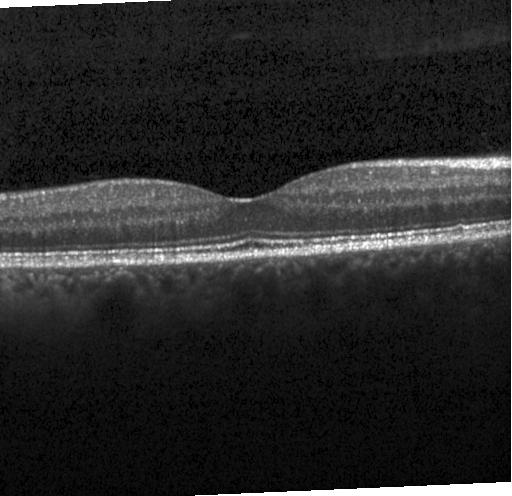
OCT line scan, instrument: Heidelberg Spectralis.
Impression: no choroidal neovascularization, no diabetic macular edema, and no drusen.